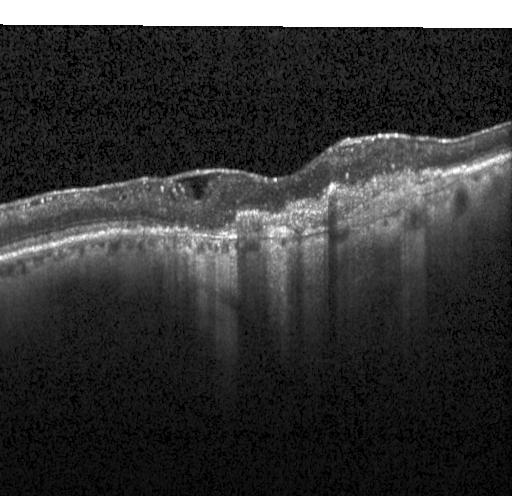 The scan shows CNV.